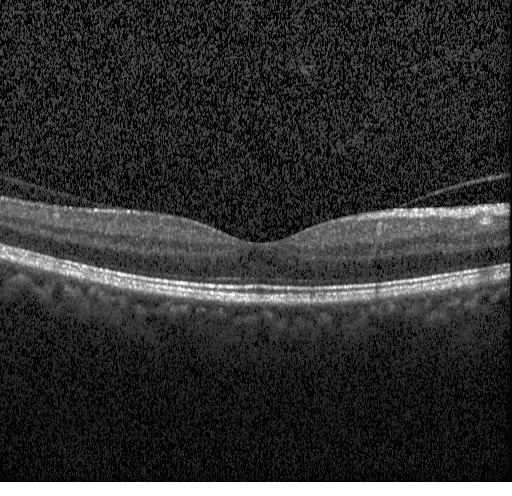 Spectral-domain OCT. Retinal OCT B-scan — Impression: neither CNV, DME, nor drusen.